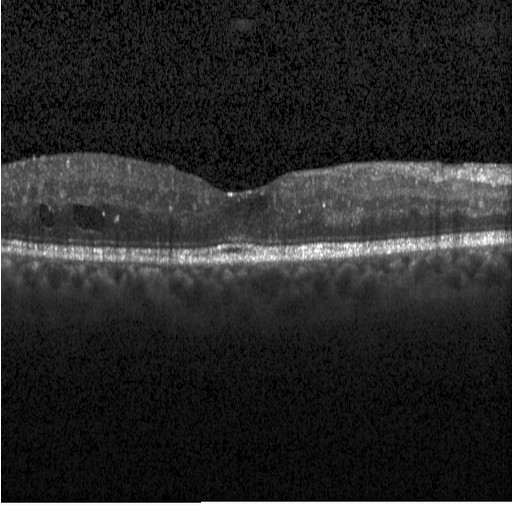

The scan shows diabetic macular edema.